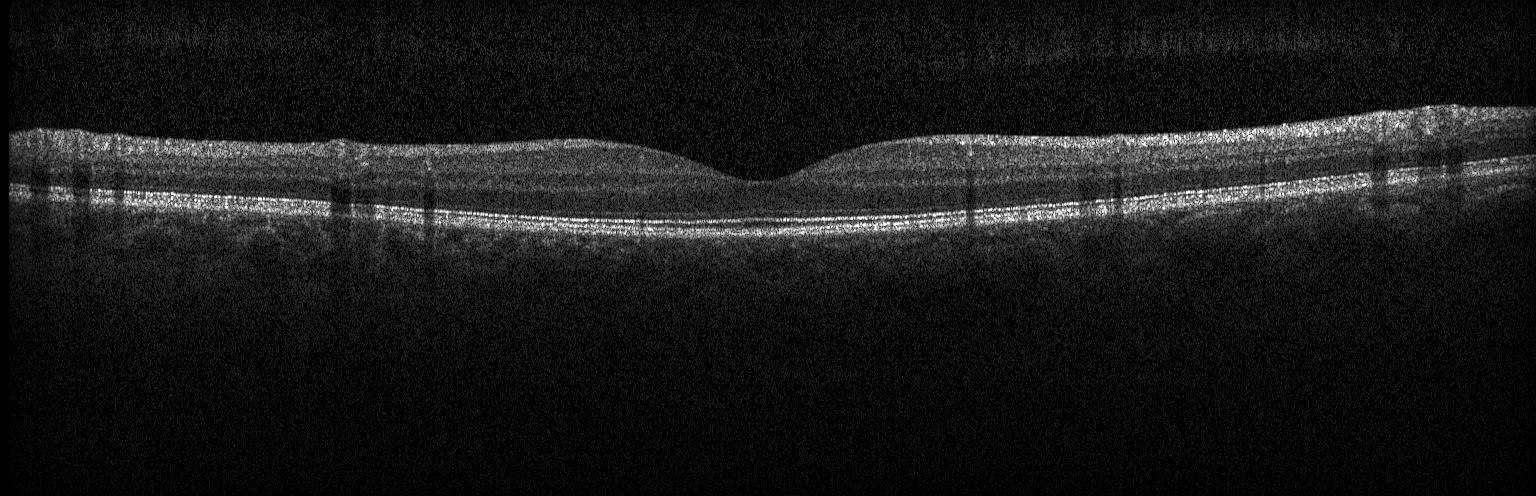
Retinal OCT cross-section
Impression: no choroidal neovascularization, no diabetic macular edema, and no drusen.